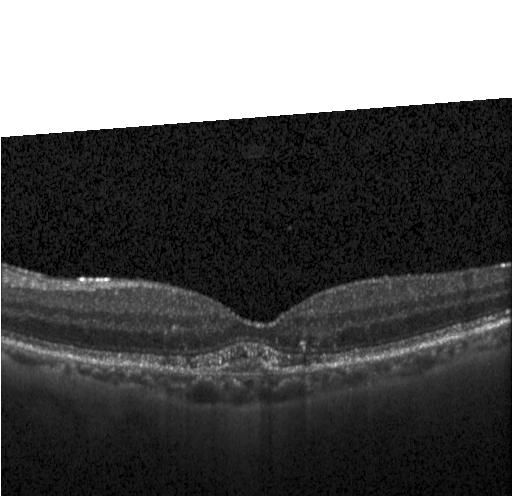
Optical coherence tomography scan — OCT finding: a choroidal neovascular membrane.